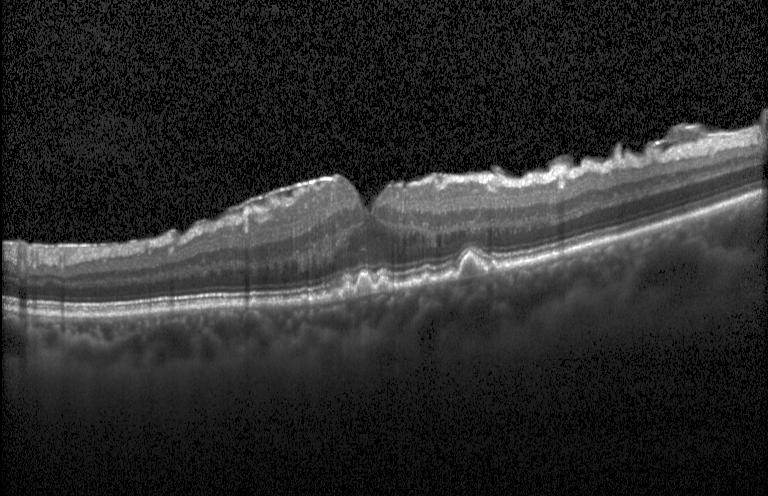
Impression: drusen.